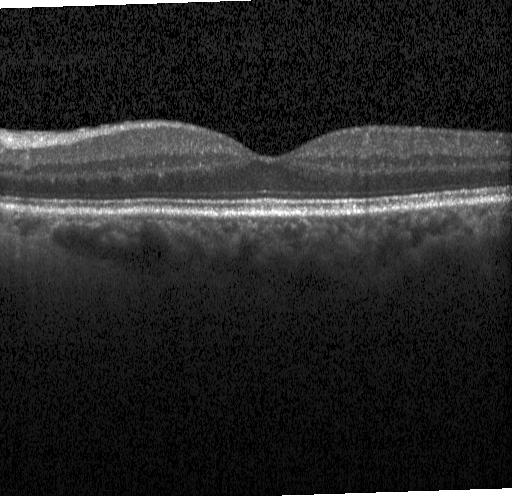
OCT scan showing neither choroidal neovascularization, diabetic macular edema, nor drusen.